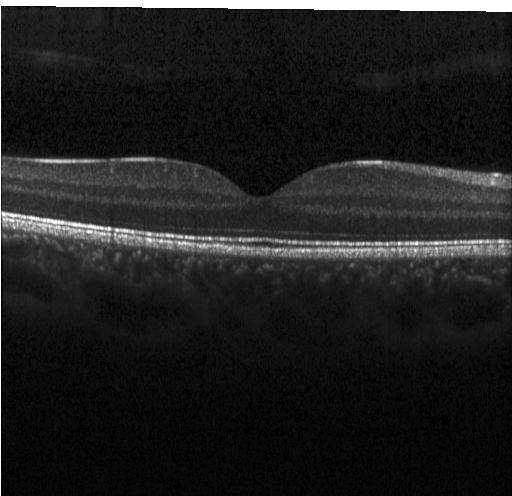
Assessment: neither choroidal neovascularization, diabetic macular edema, nor drusen.